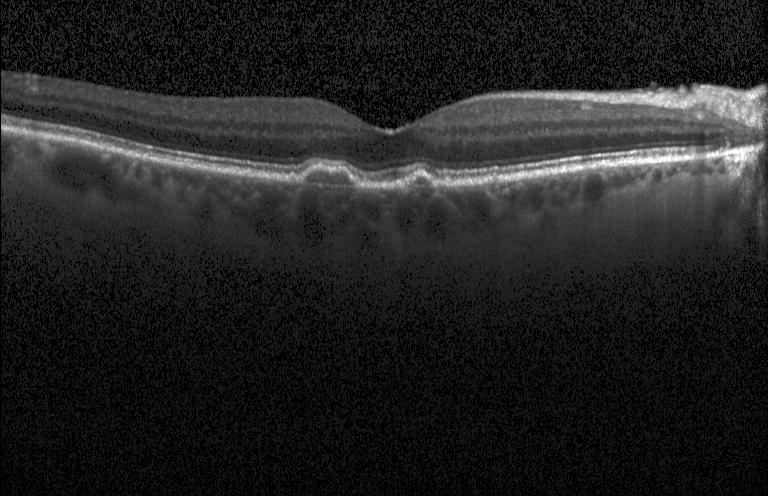

Retinal OCT cross-section; SD-OCT; macular scan; instrument: Heidelberg Spectralis
Diagnosis: sub-RPE drusenoid deposits.